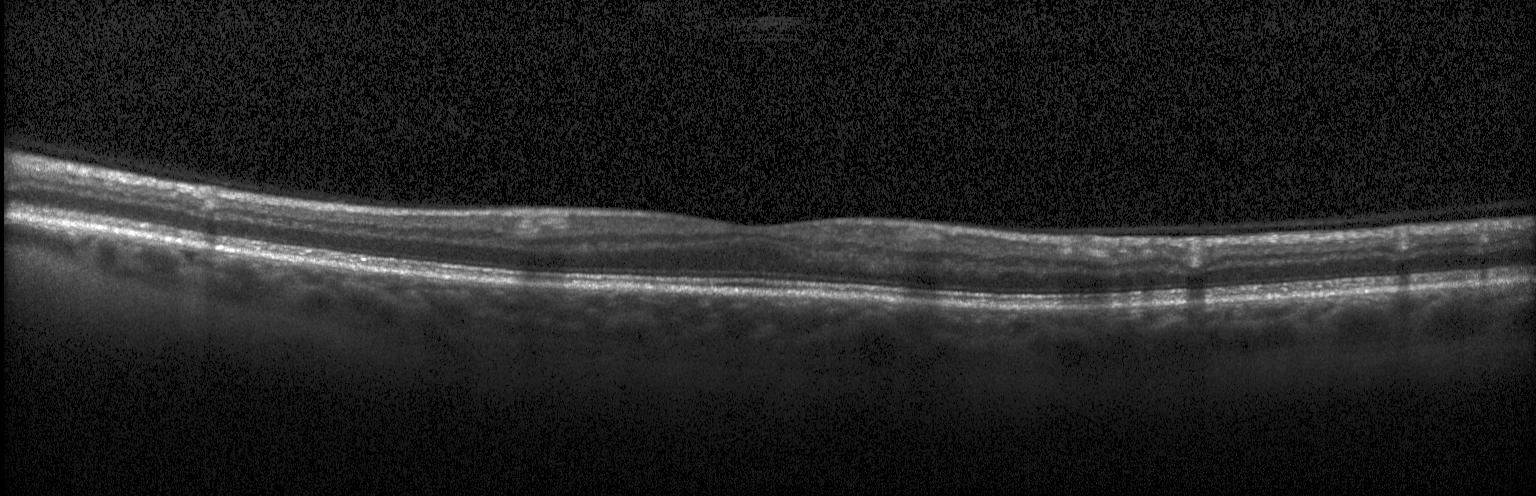

Horizontal scan through the fovea, optical coherence tomography scan. Impression: neither choroidal neovascularization, diabetic macular edema, nor drusen.